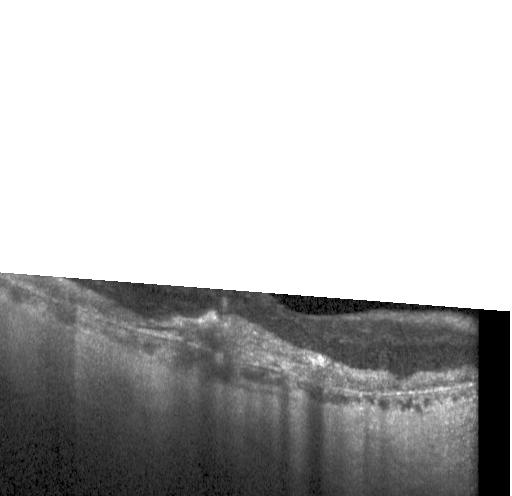
Fovea-centered. Instrument: Heidelberg Spectralis. SD-OCT. Retinal OCT cross-section. This B-scan demonstrates a choroidal neovascular membrane.